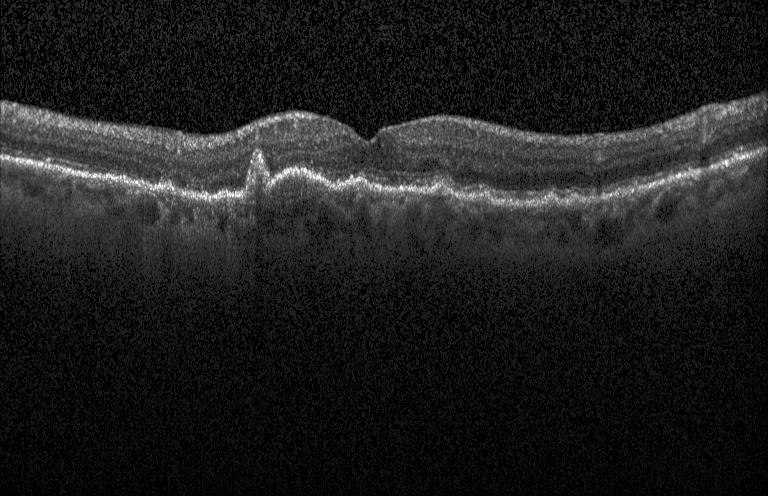
Dx: choroidal neovascularization.